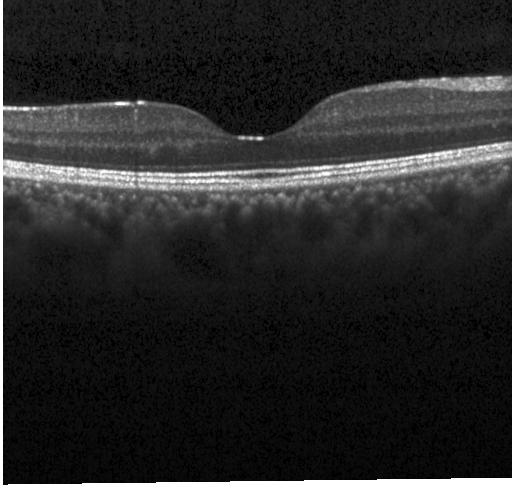

Centered on the fovea, retinal OCT B-scan — Finding: no evidence of choroidal neovascularization, diabetic macular edema, or drusen.